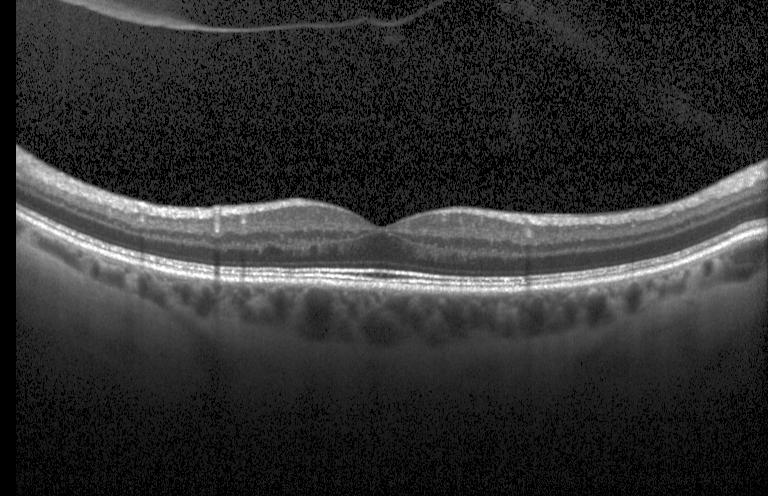 Optical coherence tomography scan
The scan shows no evidence of choroidal neovascularization, diabetic macular edema, or drusen.